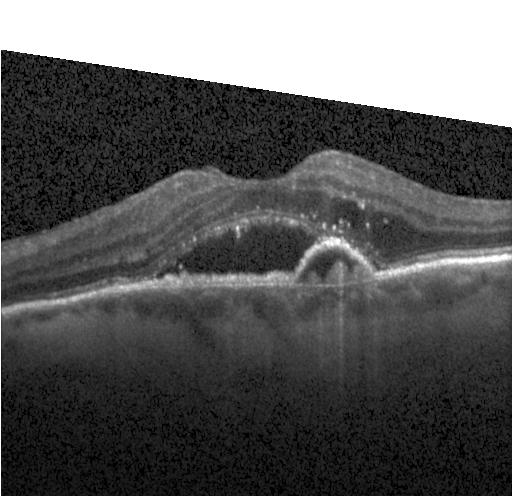

Diagnosis: a choroidal neovascular membrane.